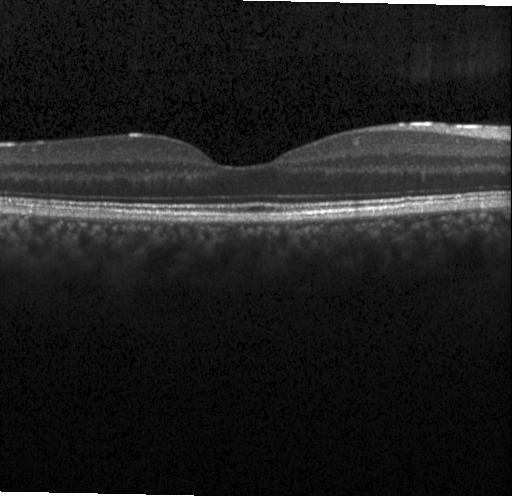
Optical coherence tomography scan
Diagnosis: neither choroidal neovascularization, diabetic macular edema, nor drusen.